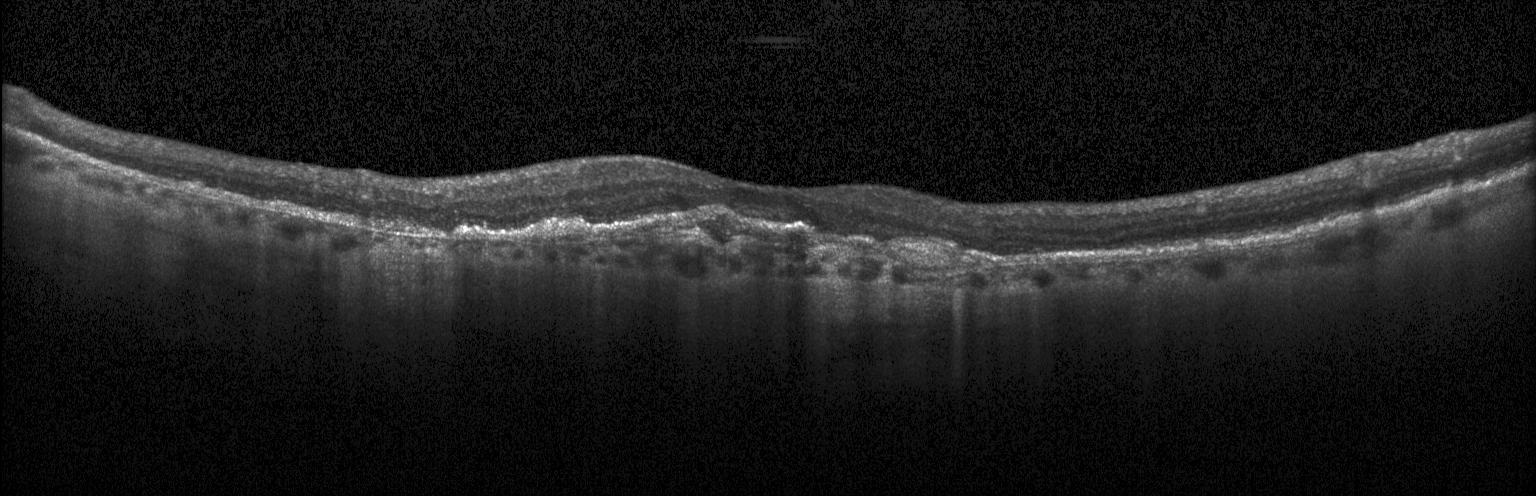

A choroidal neovascular membrane.